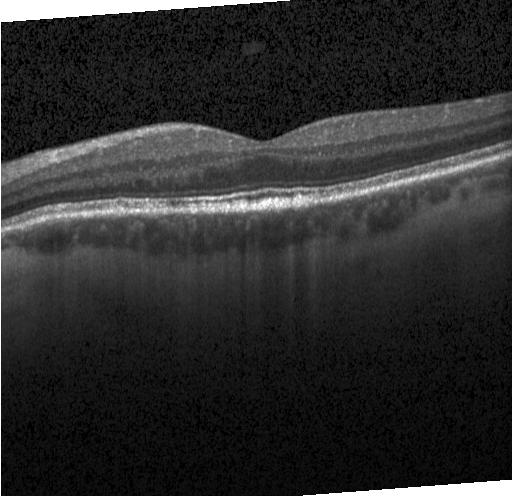

OCT B-scan showing no CNV, no DME, and no drusen.